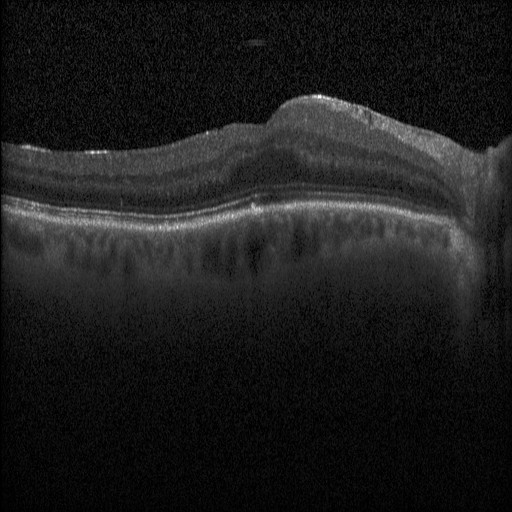 Heidelberg Spectralis OCT system, optical coherence tomography B-scan, centered on the fovea, spectral-domain OCT
Dx: diabetic macular edema.